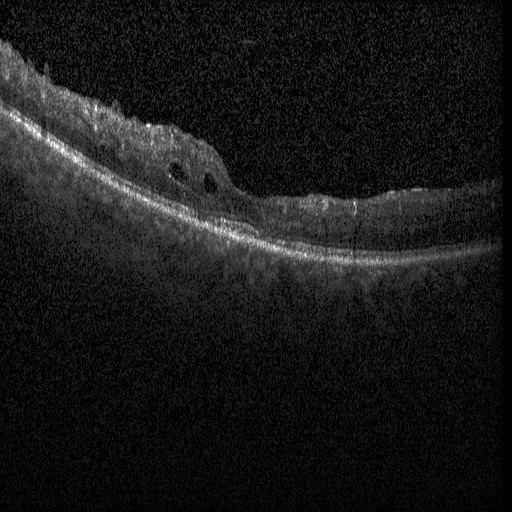
Through the macula, OCT B-scan.
Impression: DME.